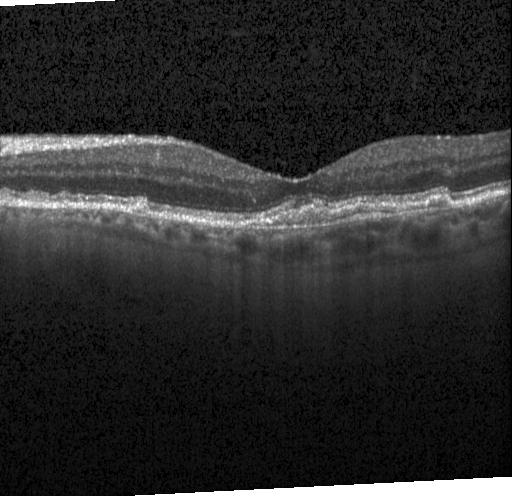

OCT line scan, SD-OCT — Finding: CNV.